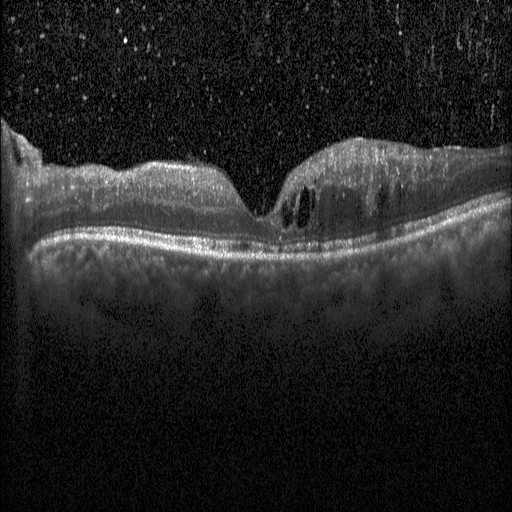
Macular OCT: diabetic macular edema.